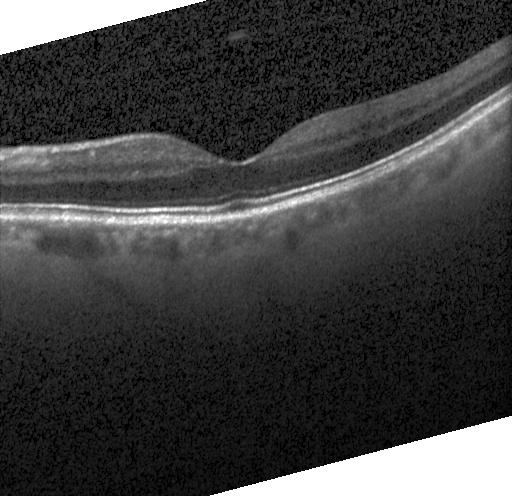

Heidelberg Spectralis OCT system · spectral-domain OCT · retinal OCT B-scan — Dx: no evidence of choroidal neovascularization, diabetic macular edema, or drusen.